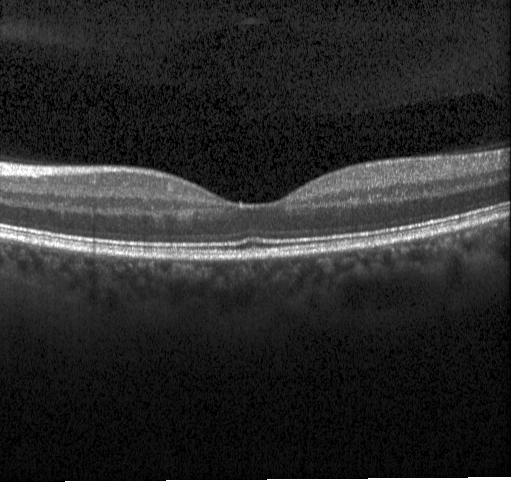
Fovea-centered, OCT B-scan, SD-OCT.
Diagnosis: no choroidal neovascularization, diabetic macular edema, or drusen.